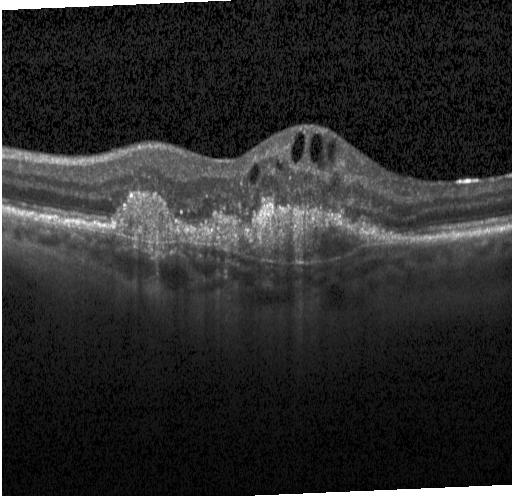

Impression: CNV.